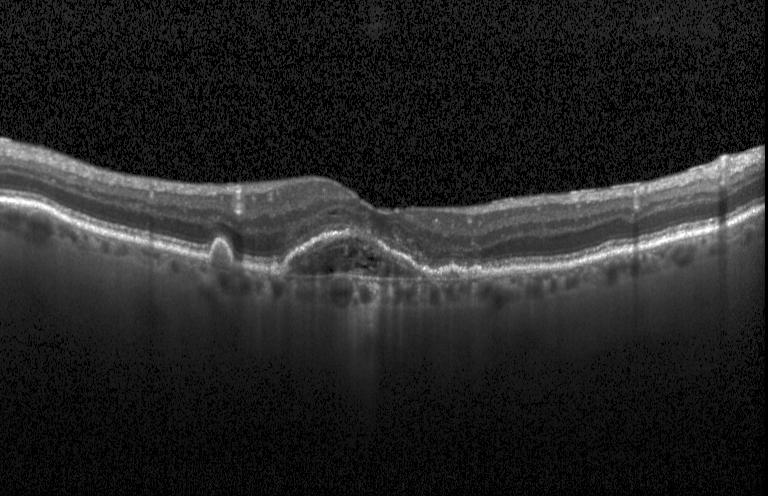
OCT finding: choroidal neovascularization.